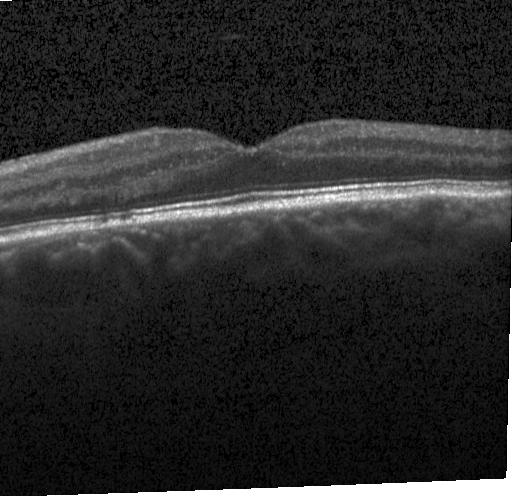 Retinal OCT B-scan · Heidelberg Spectralis OCT system · spectral-domain optical coherence tomography · horizontal scan through the fovea
Finding: no evidence of CNV, DME, or drusen.